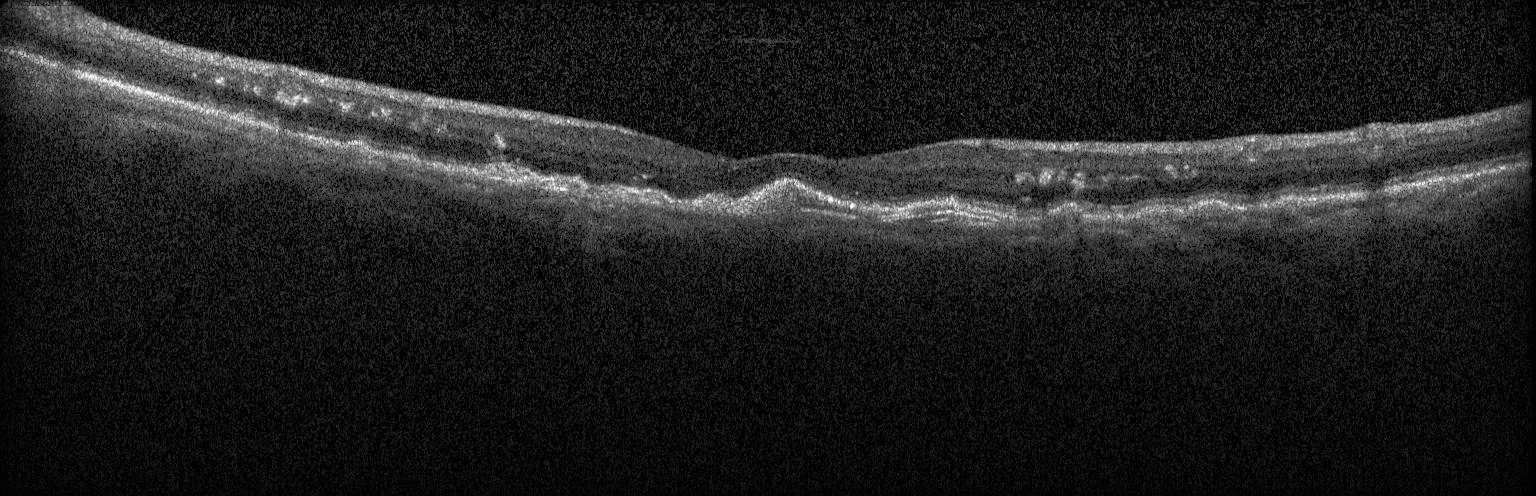
OCT B-scan showing choroidal neovascularization.